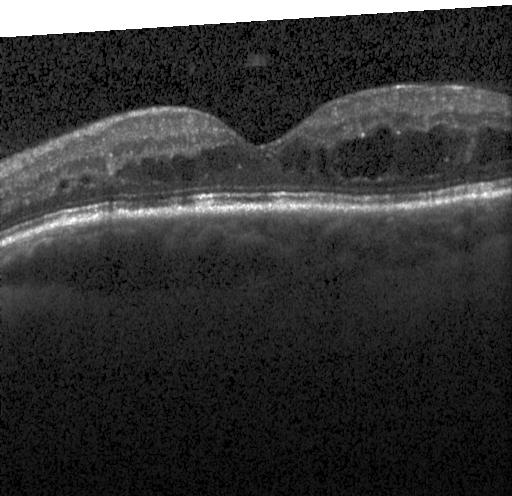

Spectral-domain optical coherence tomography, optical coherence tomography scan, Heidelberg Spectralis.
Diabetic macular edema (DME).